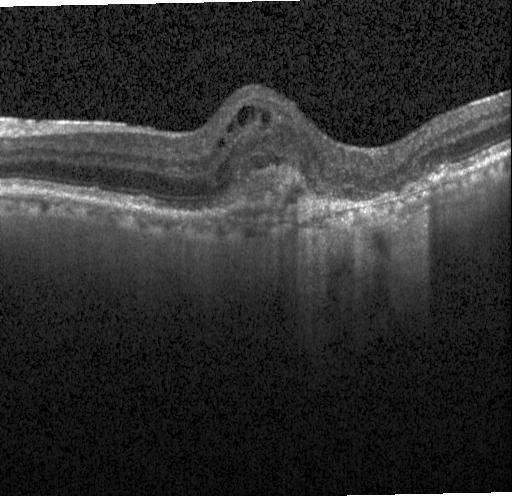 Assessment: choroidal neovascularization.